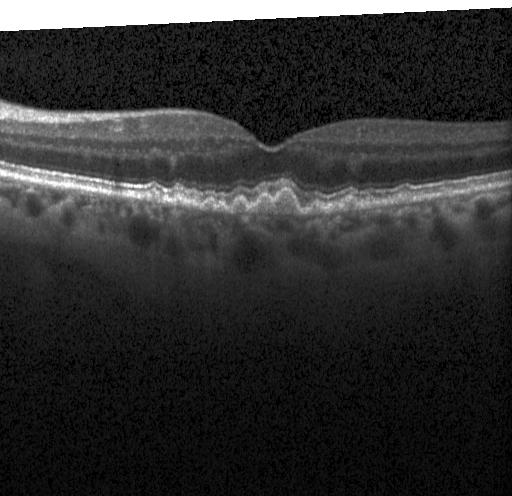

Spectral-domain OCT, acquired on a Heidelberg Spectralis, optical coherence tomography B-scan
Diagnosis: multiple drusen.